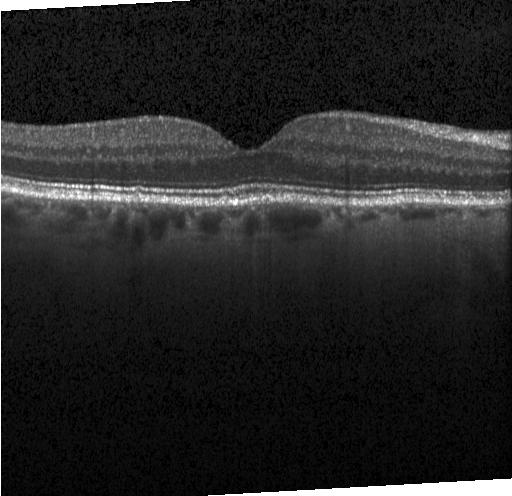 OCT line scan.
Assessment: no choroidal neovascularization, diabetic macular edema, or drusen.